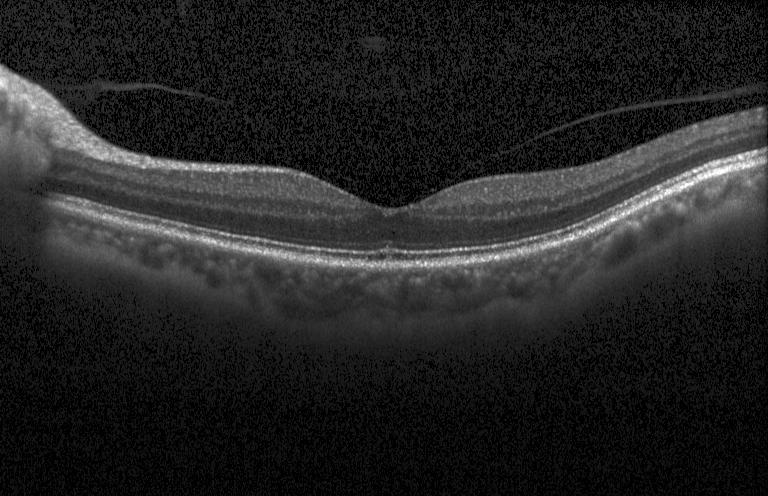 Retinal OCT cross-section. Through the macula. Spectral-domain OCT.
Assessment: no CNV, no DME, and no drusen.